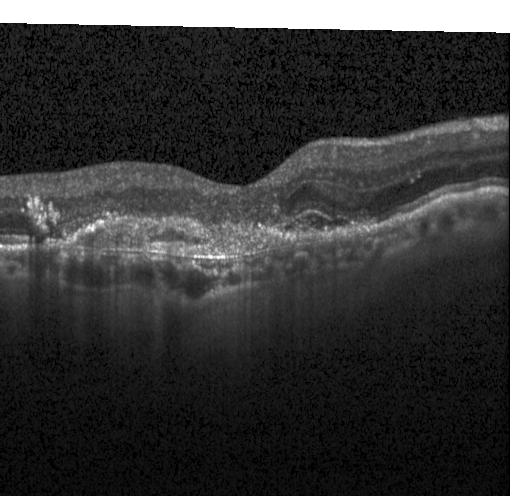 Spectral-domain optical coherence tomography. Macular scan. Heidelberg Spectralis. OCT line scan. Finding: CNV.